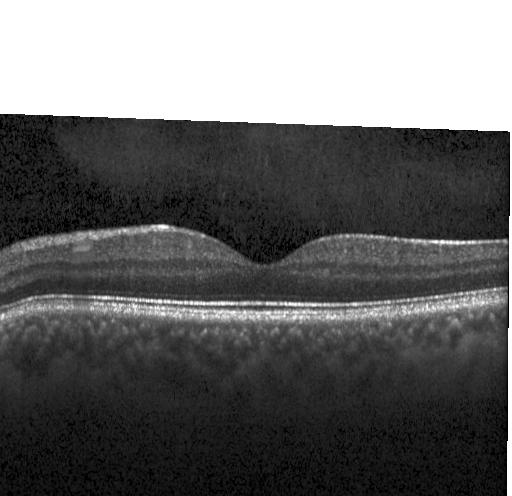 Centered on the fovea. Retinal OCT cross-section. Spectral-domain OCT — Macular OCT: no choroidal neovascularization, no diabetic macular edema, and no drusen.